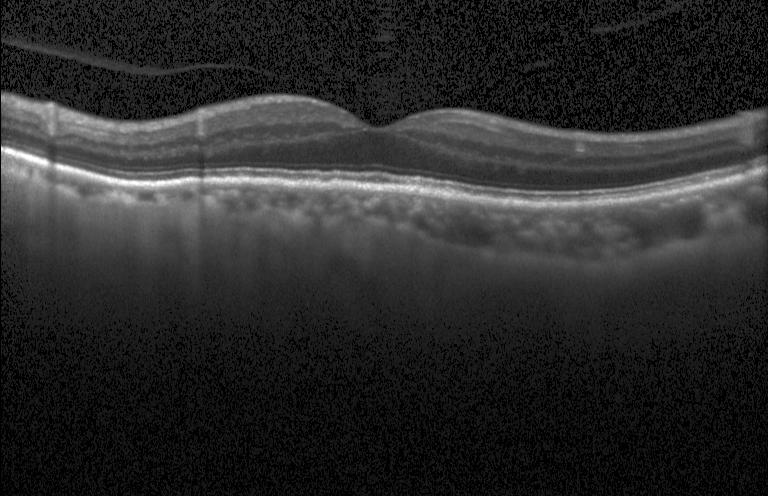
Retinal OCT B-scan.
No choroidal neovascularization, diabetic macular edema, or drusen.